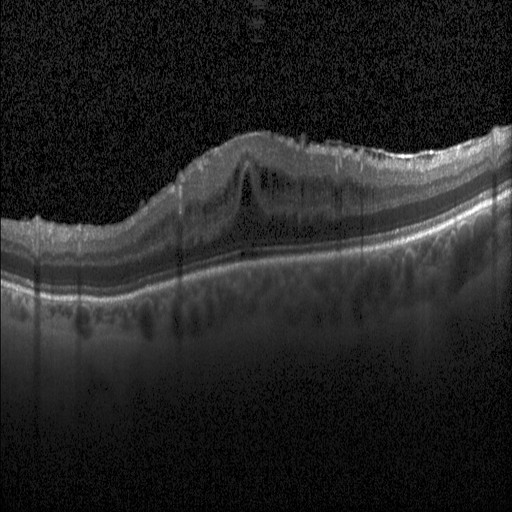

Optical coherence tomography B-scan. Horizontal scan through the fovea. Instrument: Heidelberg Spectralis. SD-OCT
Finding: diabetic macular edema.